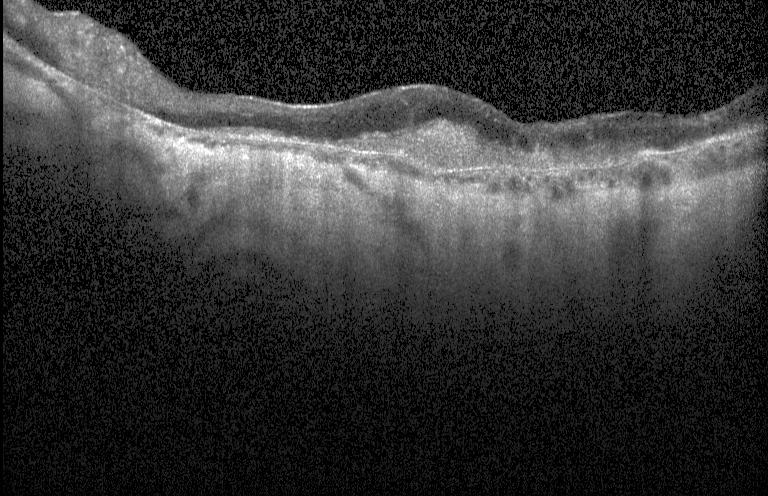
CNV.